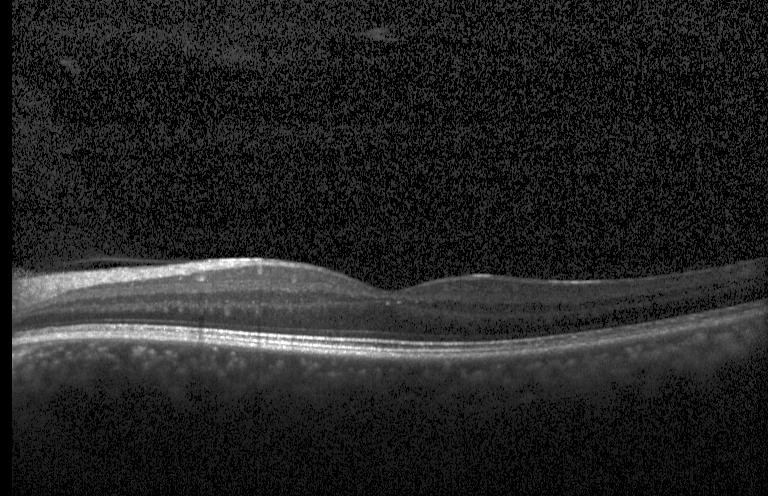

Finding: no evidence of choroidal neovascularization, diabetic macular edema, or drusen.